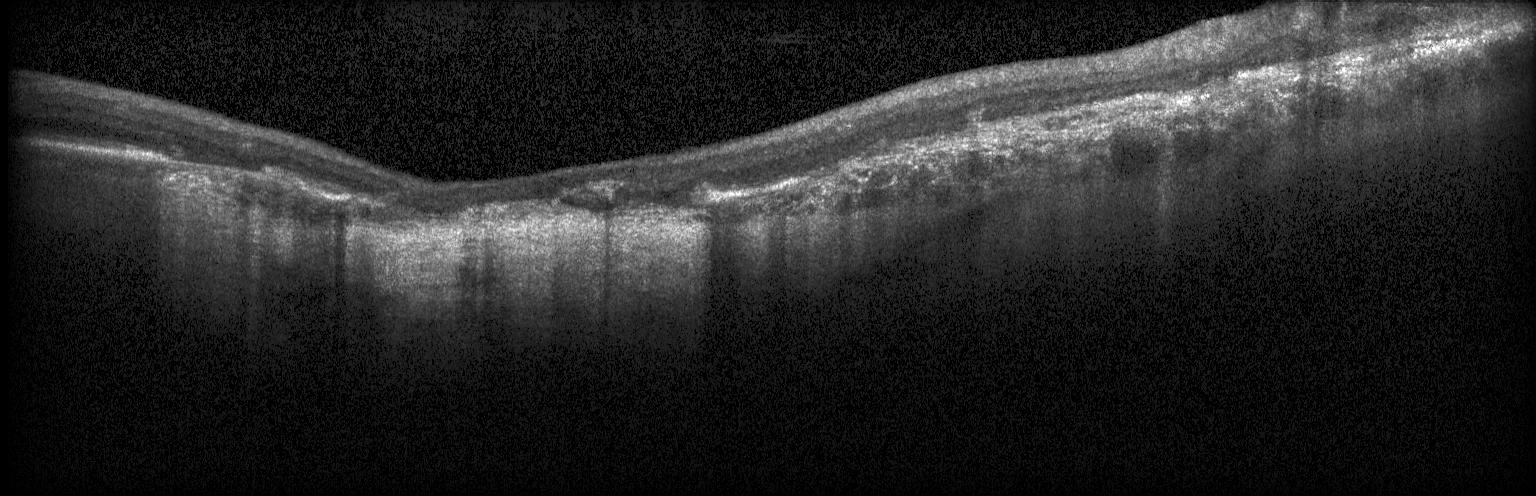
A choroidal neovascular membrane.